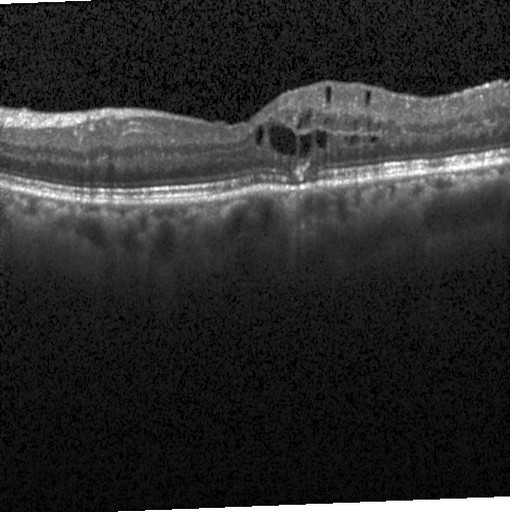 Retinal OCT B-scan, Heidelberg Spectralis OCT system
Impression: DME.